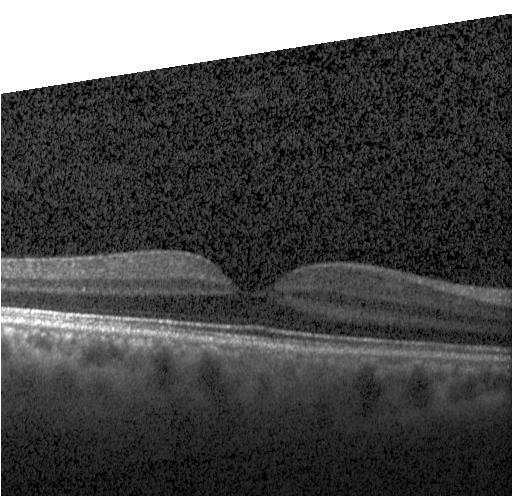

Spectral-domain OCT; optical coherence tomography B-scan.
Dx: neither CNV, DME, nor drusen.